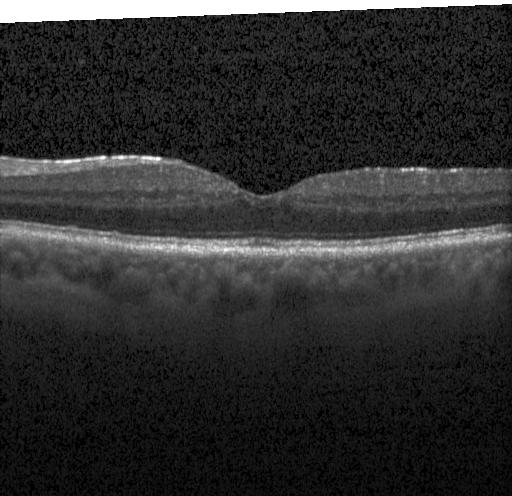
Spectral-domain optical coherence tomography · centered on the fovea · retinal OCT B-scan. Dx: no evidence of choroidal neovascularization, diabetic macular edema, or drusen.